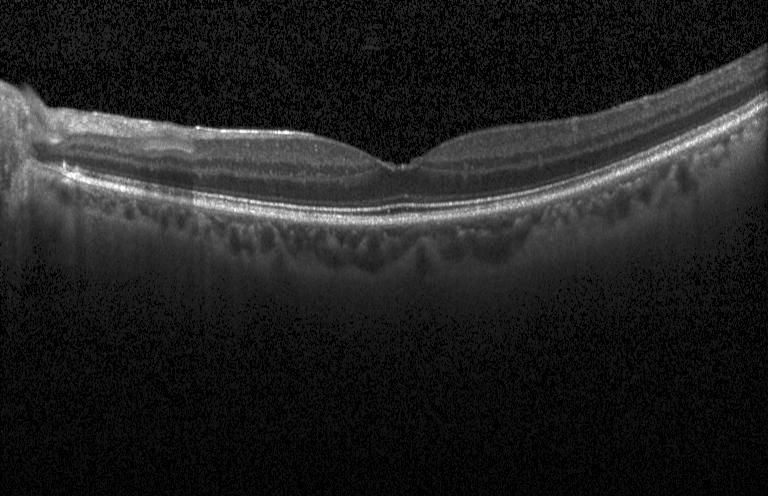
This B-scan demonstrates no evidence of choroidal neovascularization, diabetic macular edema, or drusen.